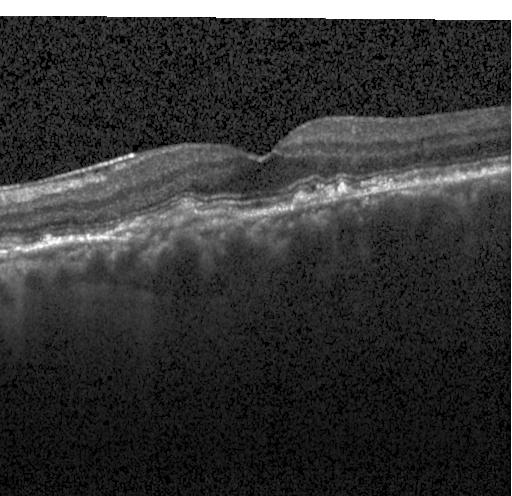
Choroidal neovascularization.